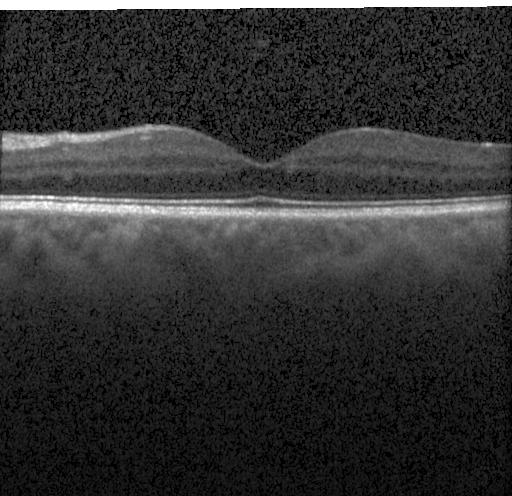

Horizontal scan through the fovea. Optical coherence tomography scan — Finding: no choroidal neovascularization, no diabetic macular edema, and no drusen.